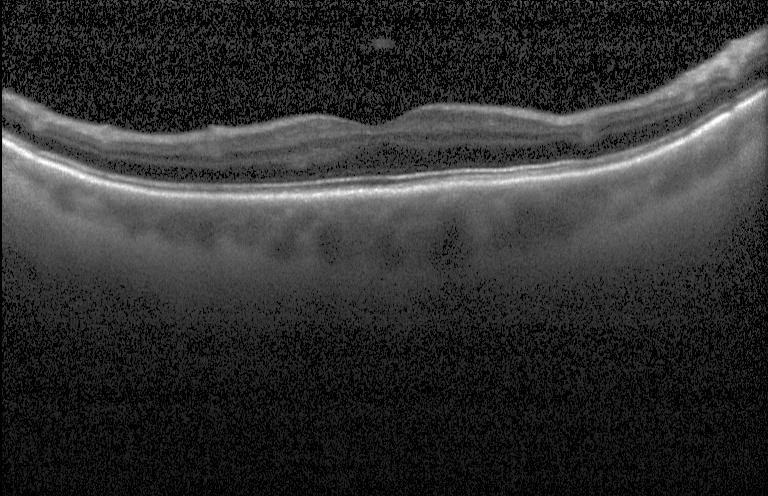
Optical coherence tomography scan · SD-OCT · acquired on a Heidelberg Spectralis · fovea-centered. OCT finding: no choroidal neovascularization, no diabetic macular edema, and no drusen.